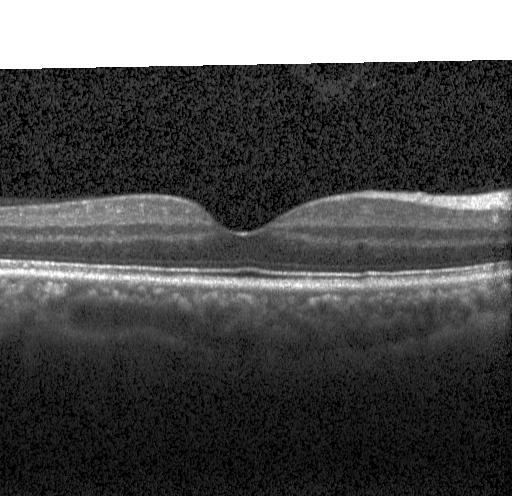
Heidelberg Spectralis OCT system, SD-OCT, fovea-centered, retinal OCT cross-section
The scan shows no evidence of choroidal neovascularization, diabetic macular edema, or drusen.